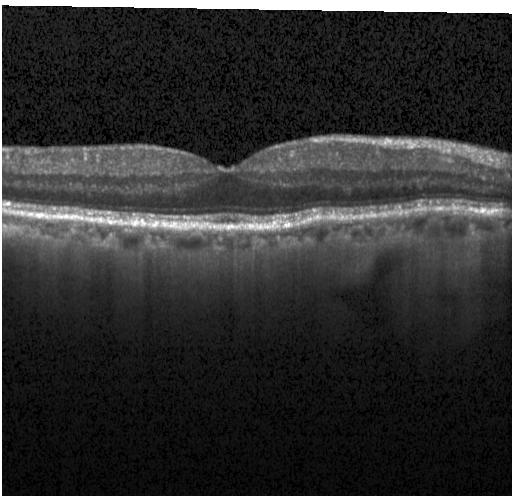
Through the macula · spectral-domain optical coherence tomography · OCT line scan · instrument: Heidelberg Spectralis.
Dx: neither choroidal neovascularization, diabetic macular edema, nor drusen.